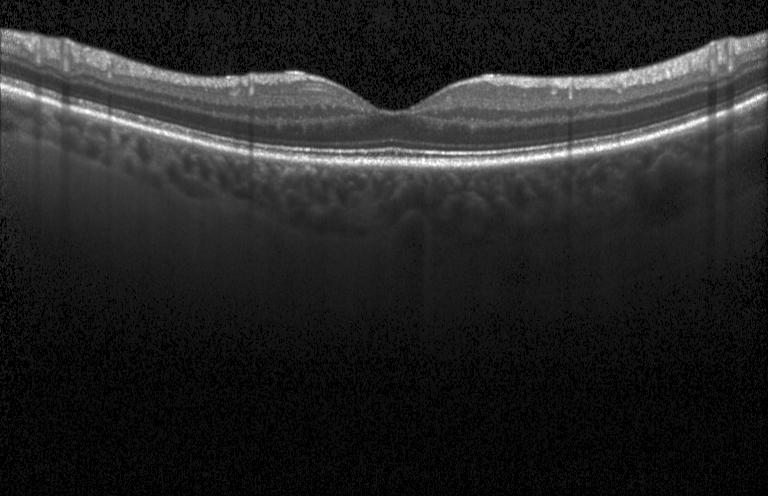
OCT B-scan — Impression: neither choroidal neovascularization, diabetic macular edema, nor drusen.